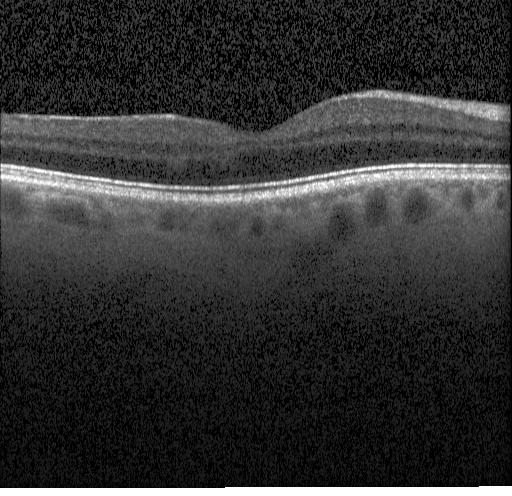
OCT line scan — Impression: no choroidal neovascularization, diabetic macular edema, or drusen.